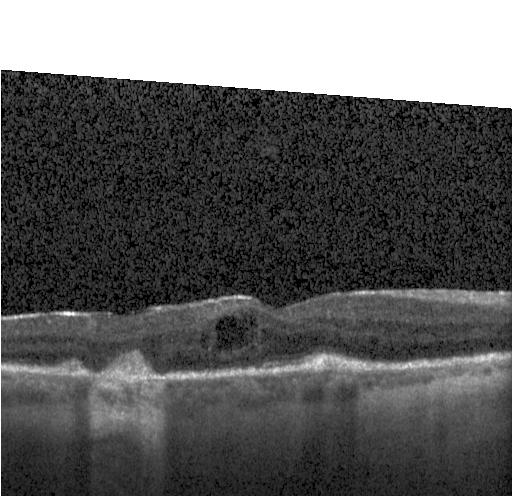 Through the macula, spectral-domain optical coherence tomography, OCT line scan, acquired on a Heidelberg Spectralis
Dx: CNV.